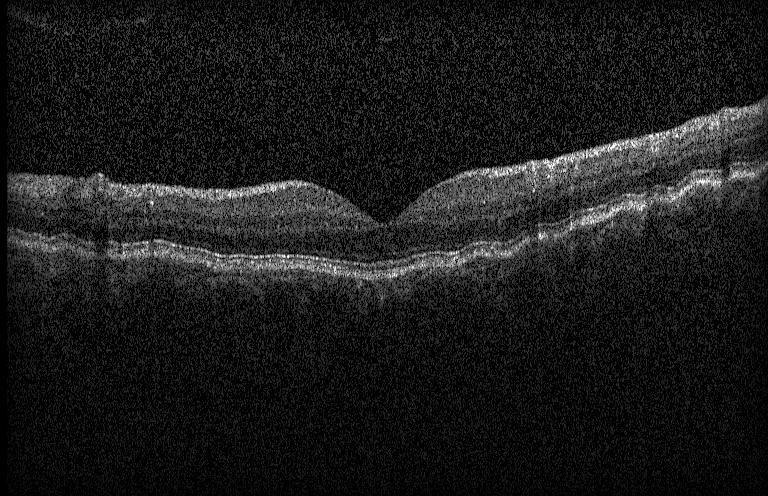

Diagnosis: drusen.